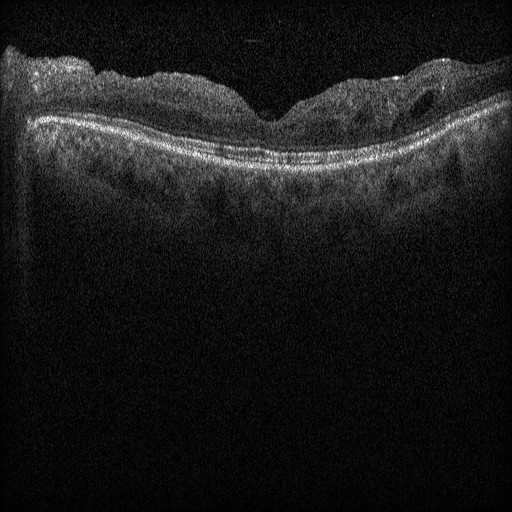 Instrument: Heidelberg Spectralis, OCT B-scan, centered on the fovea.
Dx: DME.